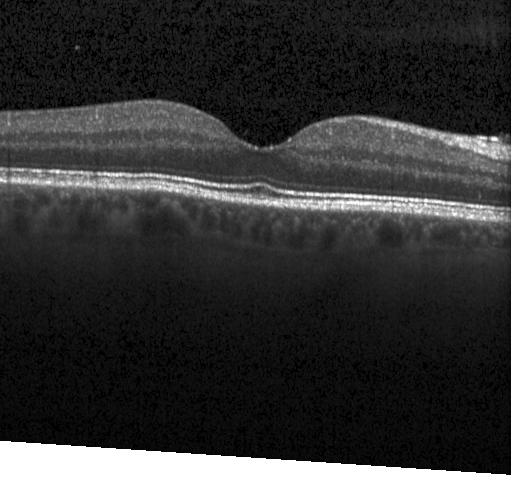

Heidelberg Spectralis OCT system, centered on the fovea, OCT B-scan, SD-OCT.
OCT finding: no CNV, no DME, and no drusen.